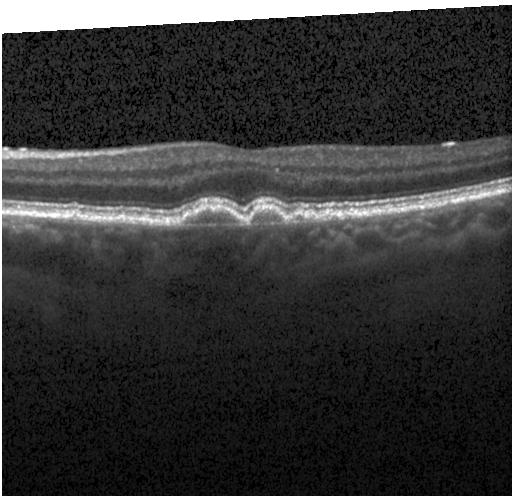

Drusen.